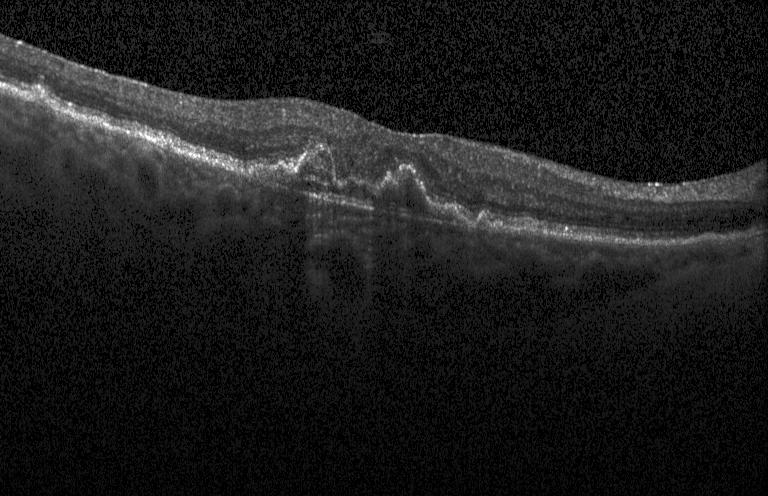 A choroidal neovascular membrane.